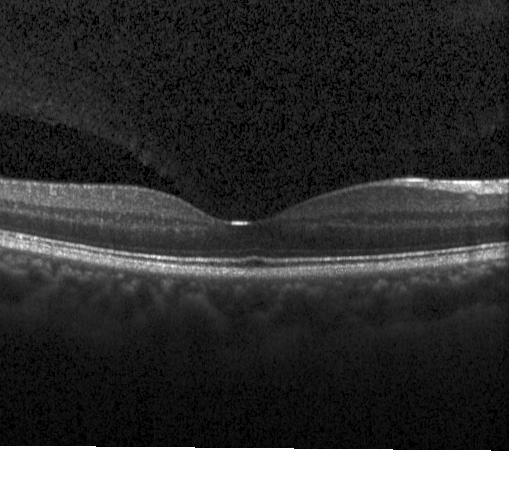

OCT scan showing no evidence of choroidal neovascularization, diabetic macular edema, or drusen.